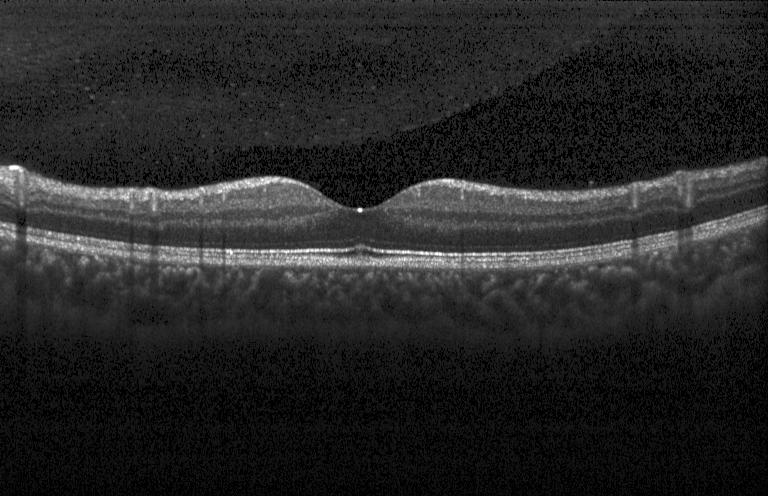 Retinal OCT B-scan · horizontal scan through the fovea — Assessment: neither choroidal neovascularization, diabetic macular edema, nor drusen.